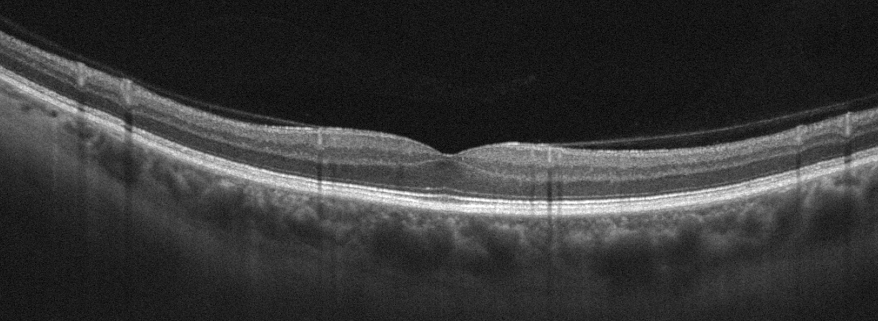
Acquired on an Optovue Avanti RTVue XR, retinal OCT B-scan. Dx: absence of AMD, DME, ERM, RAO, RVO, and vitreomacular interface disease.